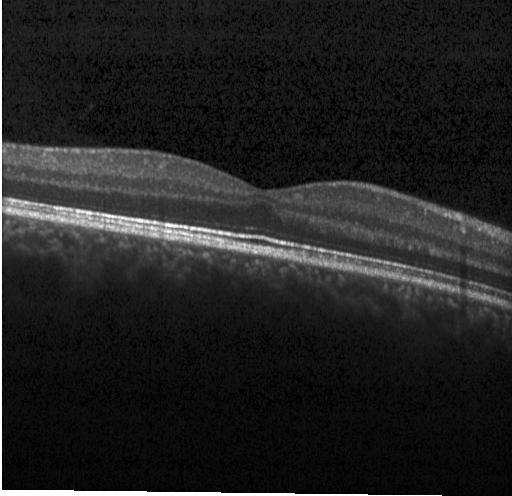 OCT line scan — Macular OCT: no choroidal neovascularization, diabetic macular edema, or drusen.